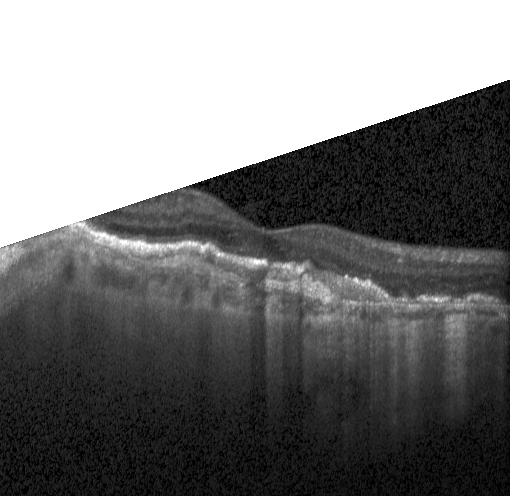 Retinal OCT cross-section.
OCT finding: a choroidal neovascular membrane.